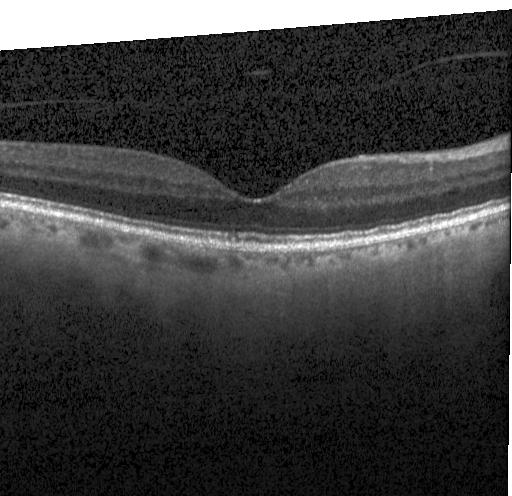
The scan shows no evidence of CNV, DME, or drusen.